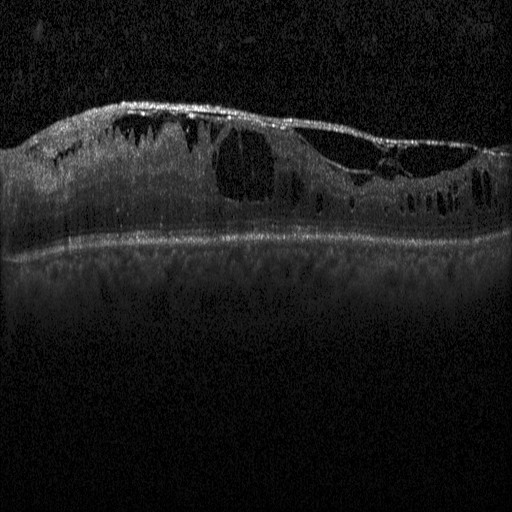 Retinal OCT cross-section, acquired on a Heidelberg Spectralis, macular scan. Diagnosis: diabetic macular edema.